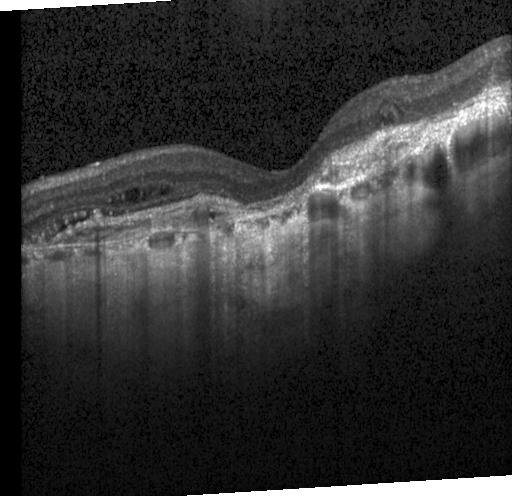
OCT B-scan.
Diagnosis: a choroidal neovascular membrane.